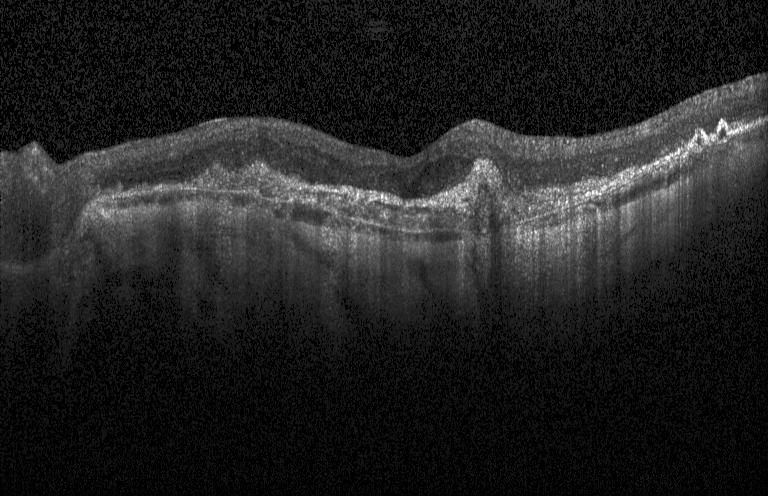 Fovea-centered; OCT line scan
Impression: CNV.